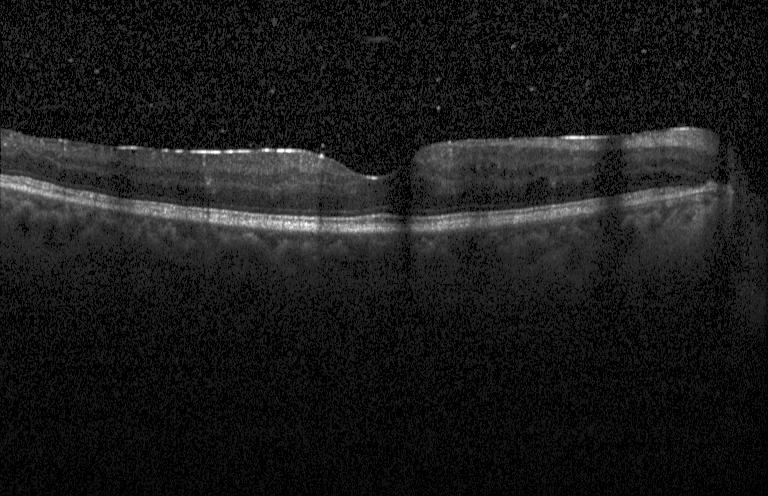

Through the macula, Heidelberg Spectralis, optical coherence tomography scan, spectral-domain optical coherence tomography.
Finding: no choroidal neovascularization, no diabetic macular edema, and no drusen.